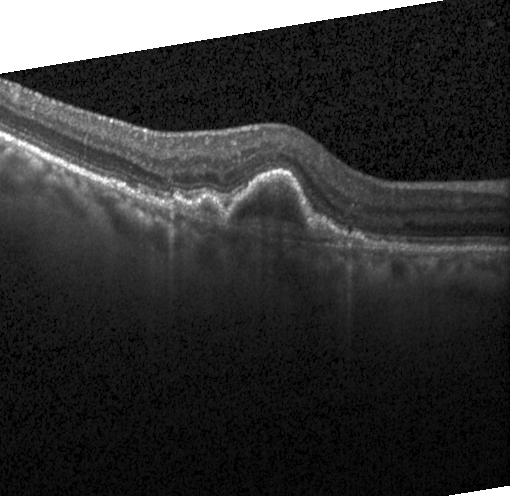

Retinal OCT B-scan · macular scan · spectral-domain OCT · acquired on a Heidelberg Spectralis.
Finding: a choroidal neovascular membrane.